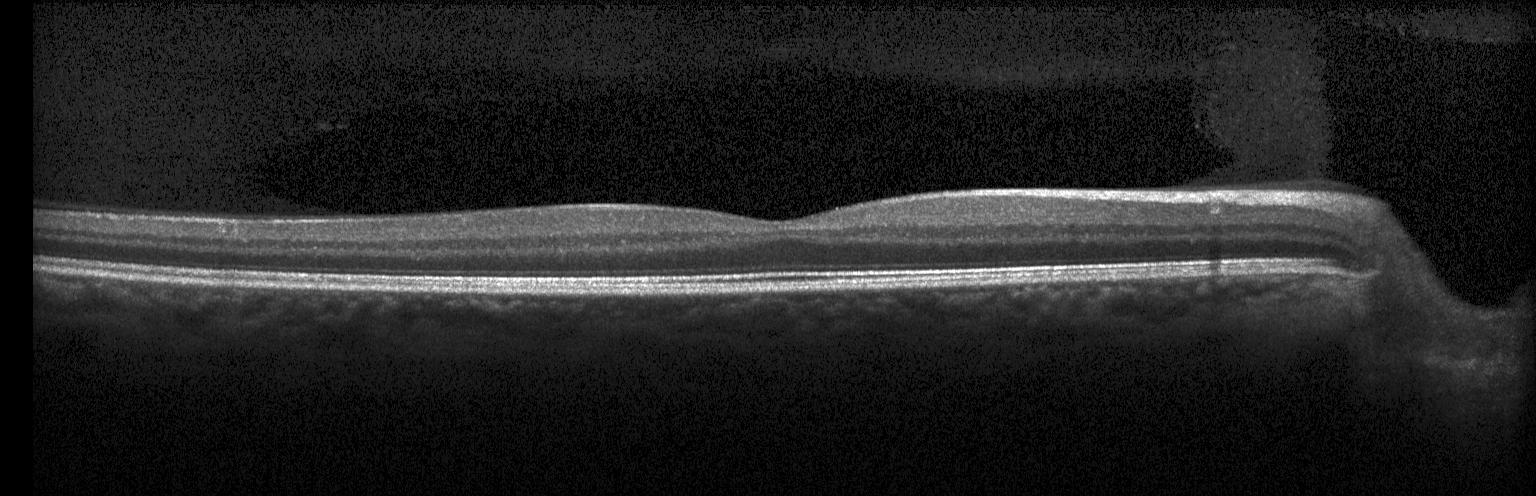
Heidelberg Spectralis · optical coherence tomography scan
Diagnosis: no choroidal neovascularization, diabetic macular edema, or drusen.